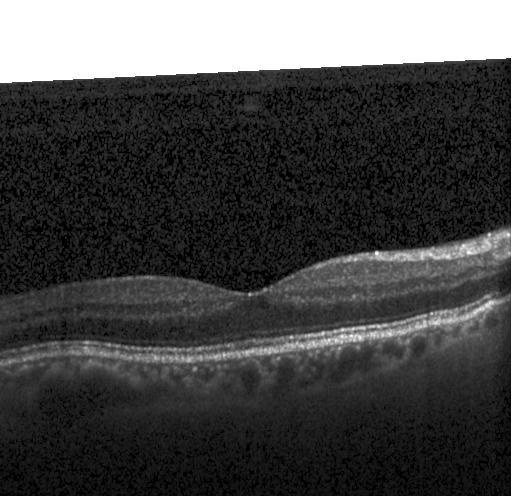
Finding: no choroidal neovascularization, no diabetic macular edema, and no drusen.